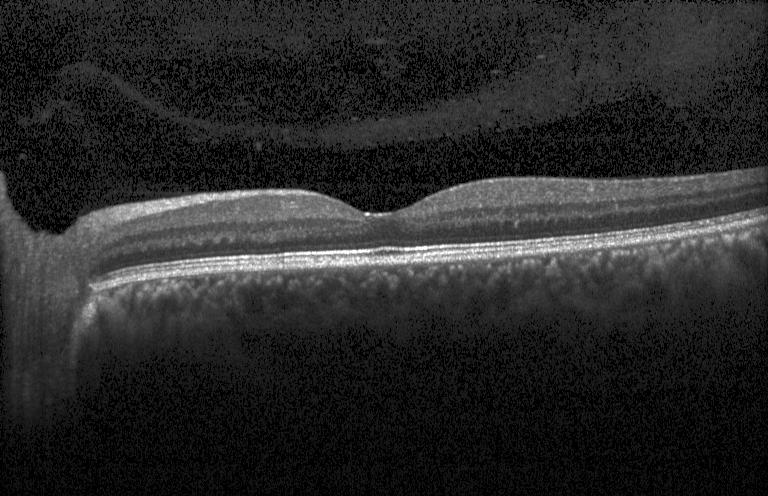

Impression: neither CNV, DME, nor drusen.